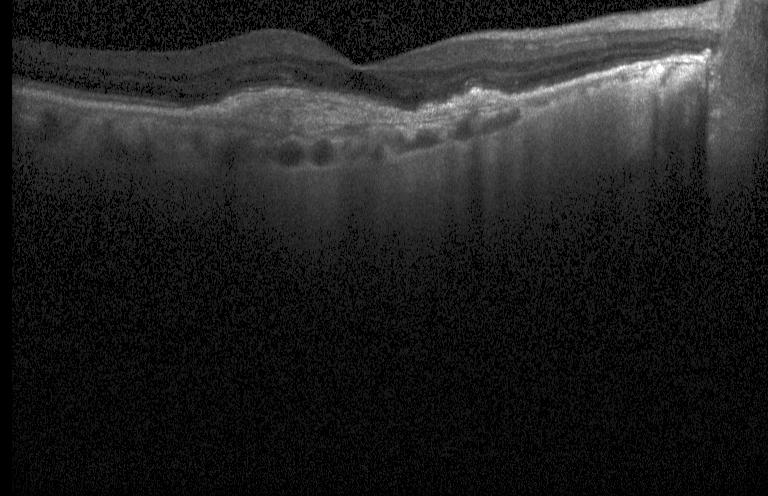

OCT B-scan · fovea-centered · Heidelberg Spectralis.
Macular OCT: a choroidal neovascular membrane.